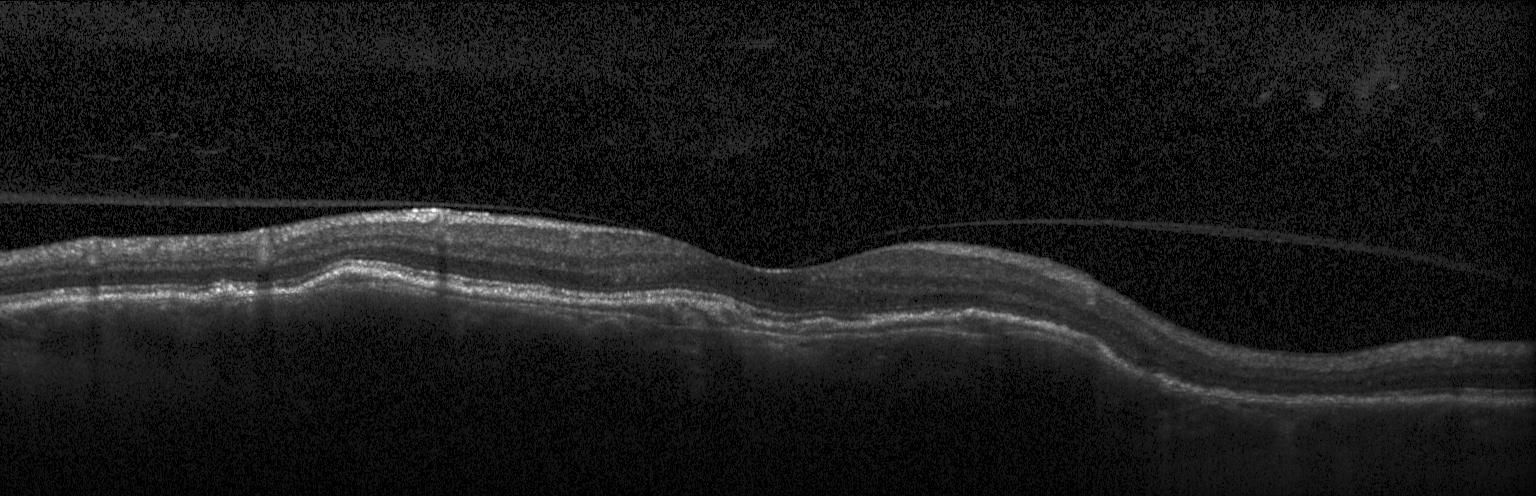 Retinal OCT B-scan. Horizontal scan through the fovea.
Diagnosis: a choroidal neovascular membrane.